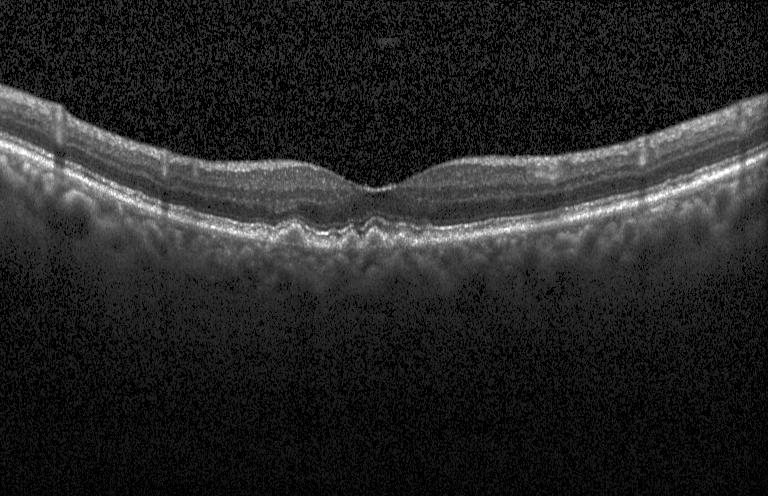

Retinal OCT B-scan.
Sub-RPE drusenoid deposits.